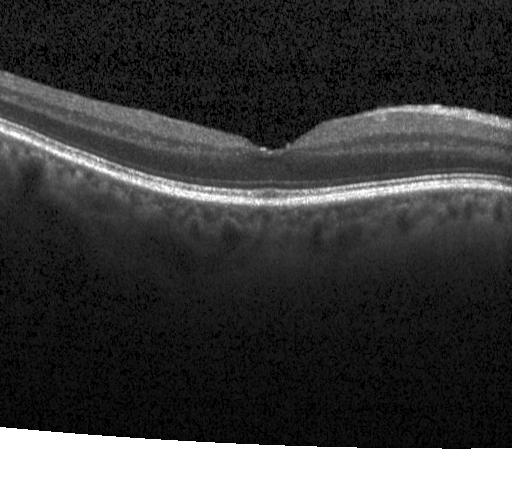 No choroidal neovascularization, no diabetic macular edema, and no drusen.